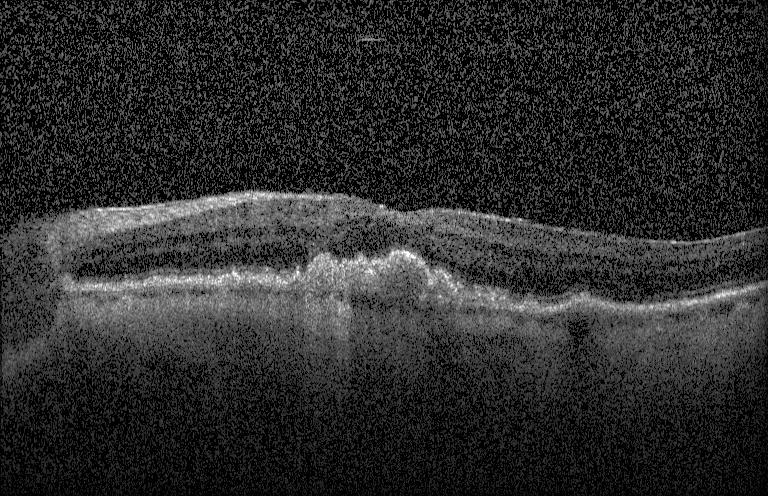
Centered on the fovea · spectral-domain optical coherence tomography · OCT line scan — Dx: choroidal neovascularization.